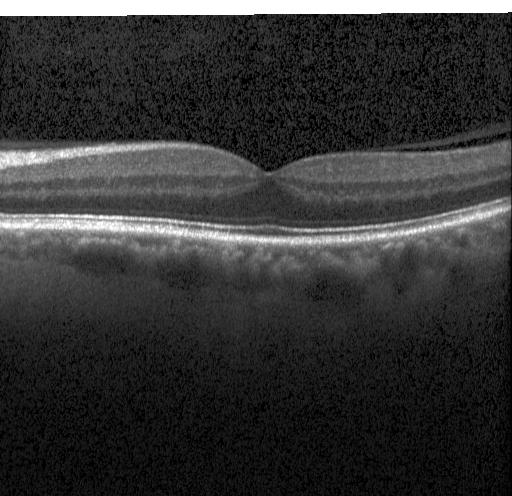 OCT line scan; centered on the fovea; Heidelberg Spectralis — No evidence of CNV, DME, or drusen.